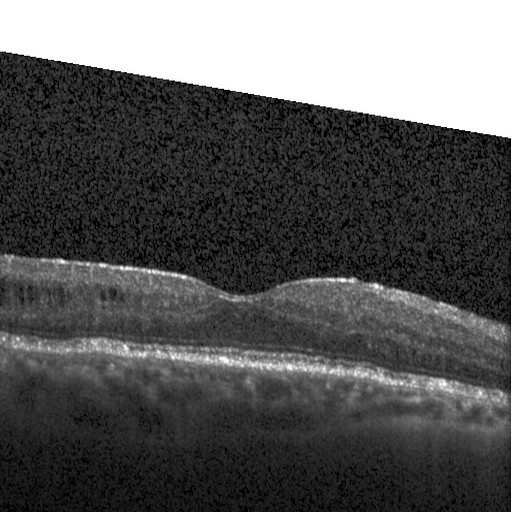 OCT B-scan showing DME.